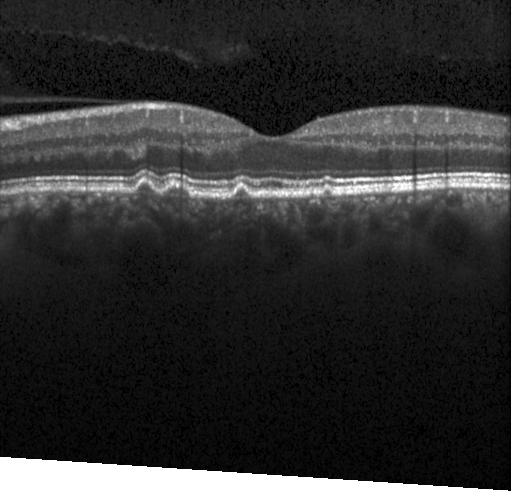 SD-OCT; optical coherence tomography scan; horizontal scan through the fovea; Heidelberg Spectralis OCT system.
Diagnosis: drusen.